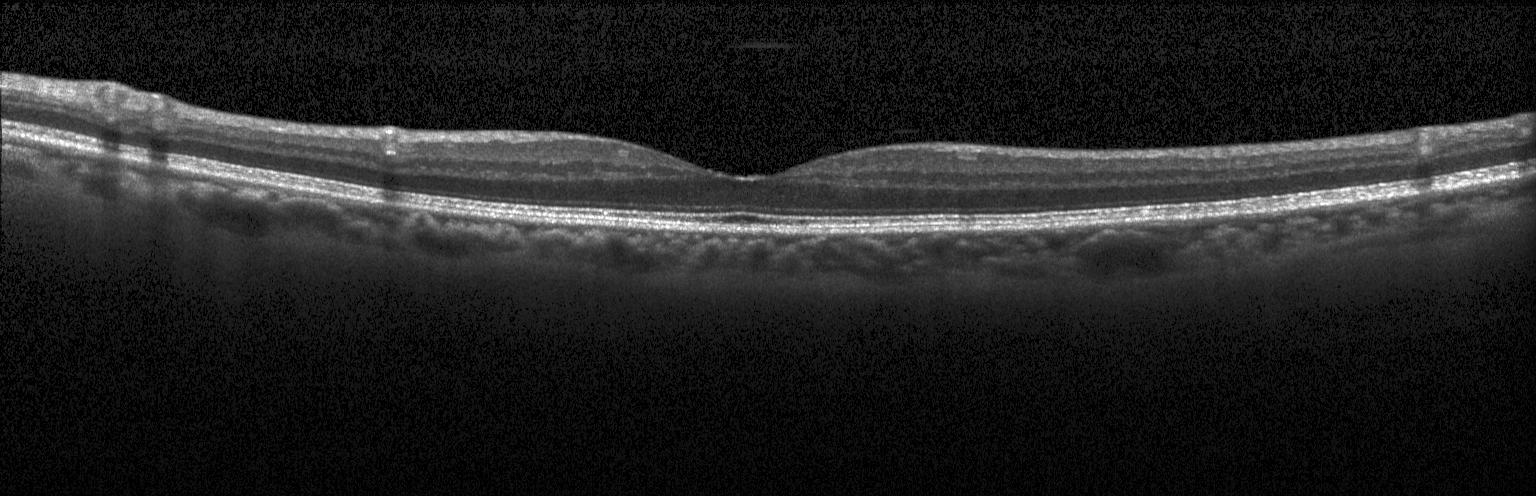

Retinal OCT cross-section showing no evidence of CNV, DME, or drusen.